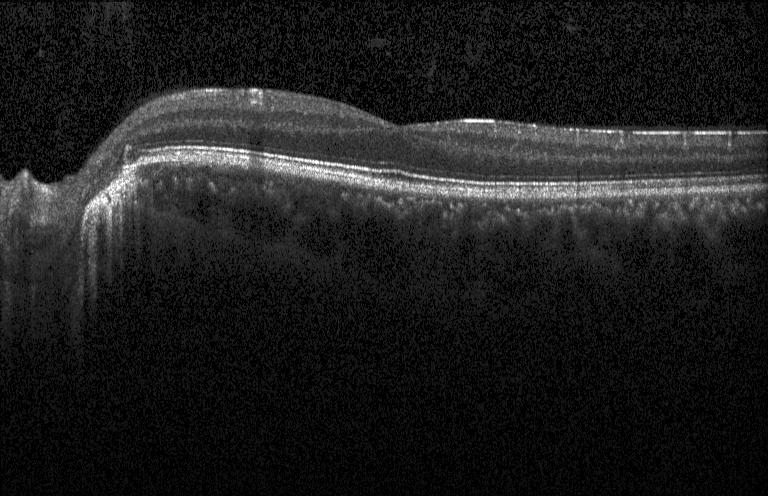
OCT B-scan
Finding: no choroidal neovascularization, diabetic macular edema, or drusen.